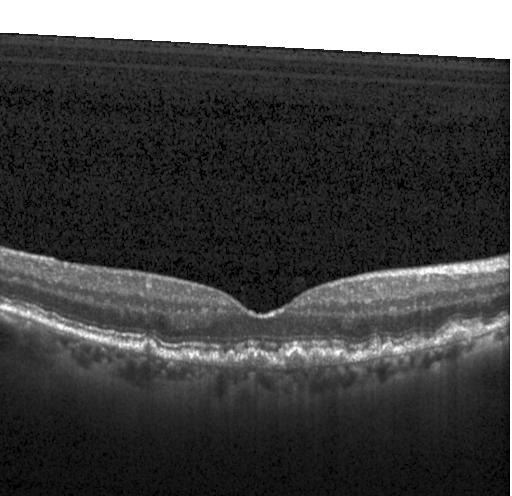

Retinal OCT B-scan.
Macular OCT: sub-RPE drusenoid deposits.